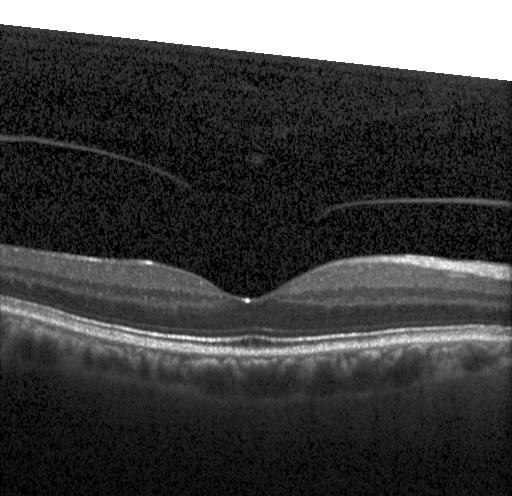 OCT line scan, horizontal scan through the fovea, Heidelberg Spectralis OCT system
Diagnosis: neither CNV, DME, nor drusen.